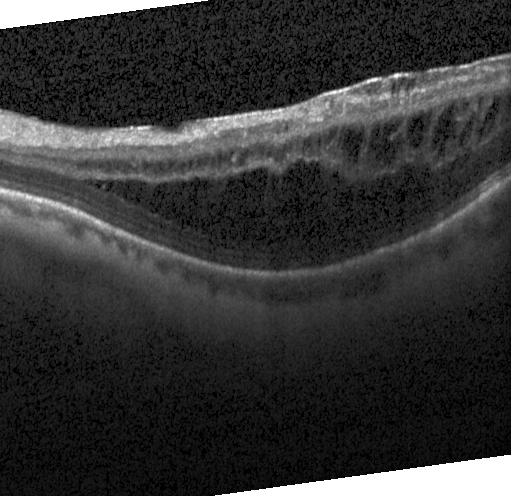 Diagnosis: diabetic macular edema.